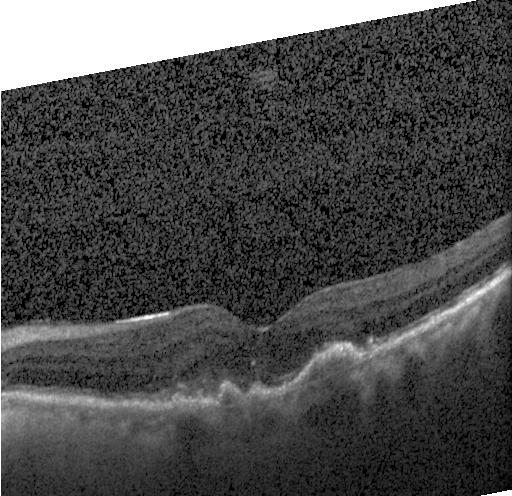 SD-OCT · centered on the fovea · optical coherence tomography B-scan — A choroidal neovascular membrane.